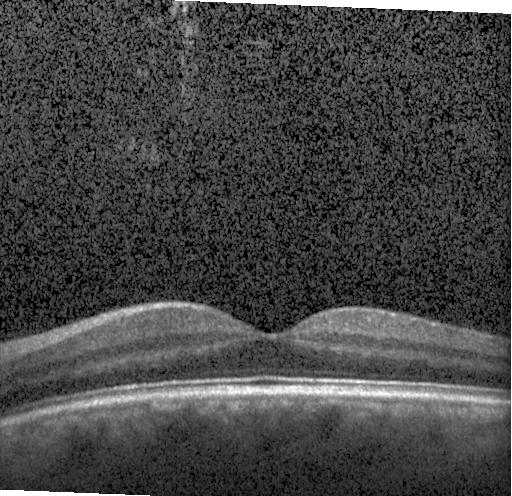

Assessment: neither CNV, DME, nor drusen.